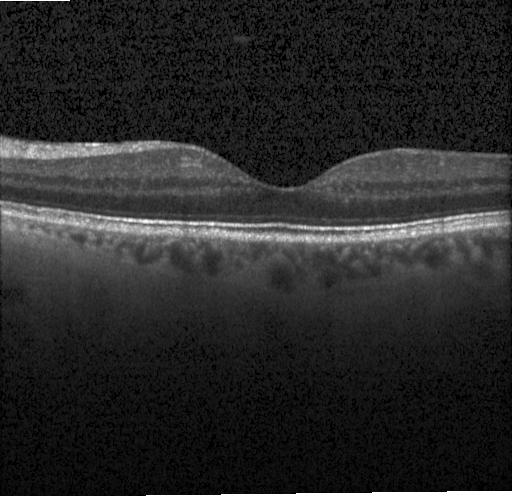
Optical coherence tomography B-scan. Impression: neither CNV, DME, nor drusen.